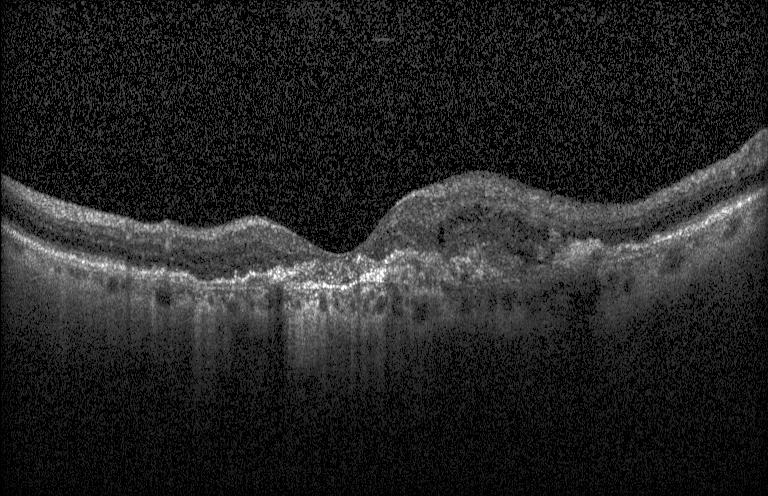
Retinal OCT B-scan. Heidelberg Spectralis.
Assessment: choroidal neovascularization.